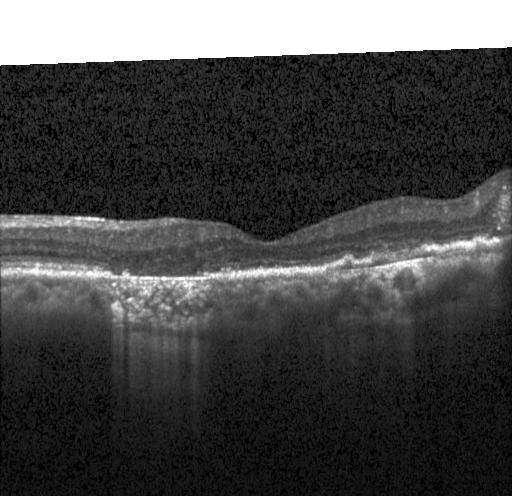
Optical coherence tomography B-scan. Choroidal neovascularization (CNV).